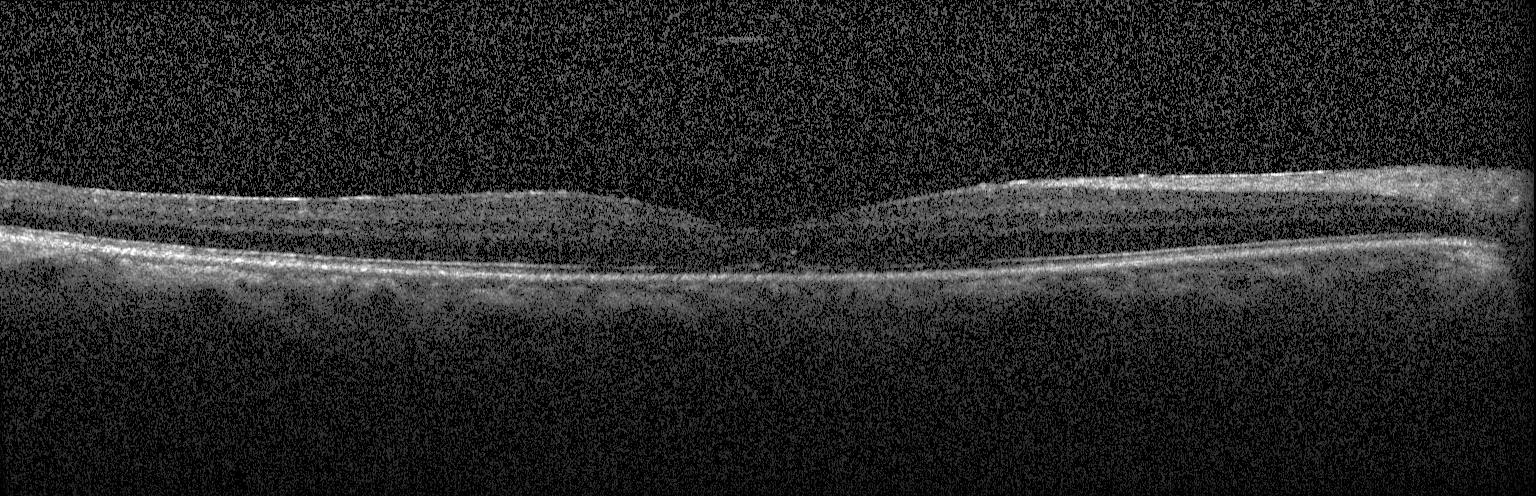
Diagnosis: no evidence of choroidal neovascularization, diabetic macular edema, or drusen.